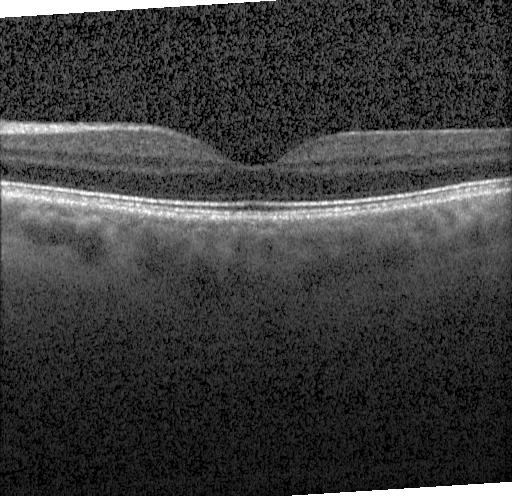

Impression: no evidence of choroidal neovascularization, diabetic macular edema, or drusen.